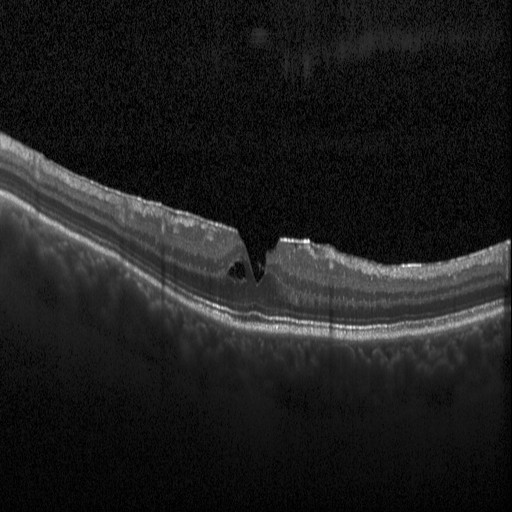
Spectral-domain OCT, horizontal scan through the fovea, optical coherence tomography scan, Heidelberg Spectralis
Assessment: diabetic macular edema.